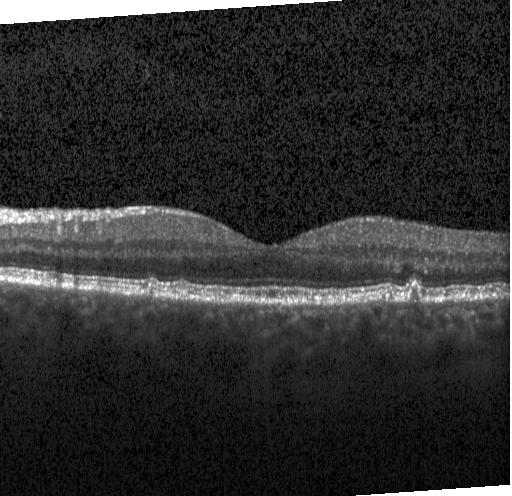

Optical coherence tomography B-scan · horizontal scan through the fovea
Dx: sub-RPE drusenoid deposits.